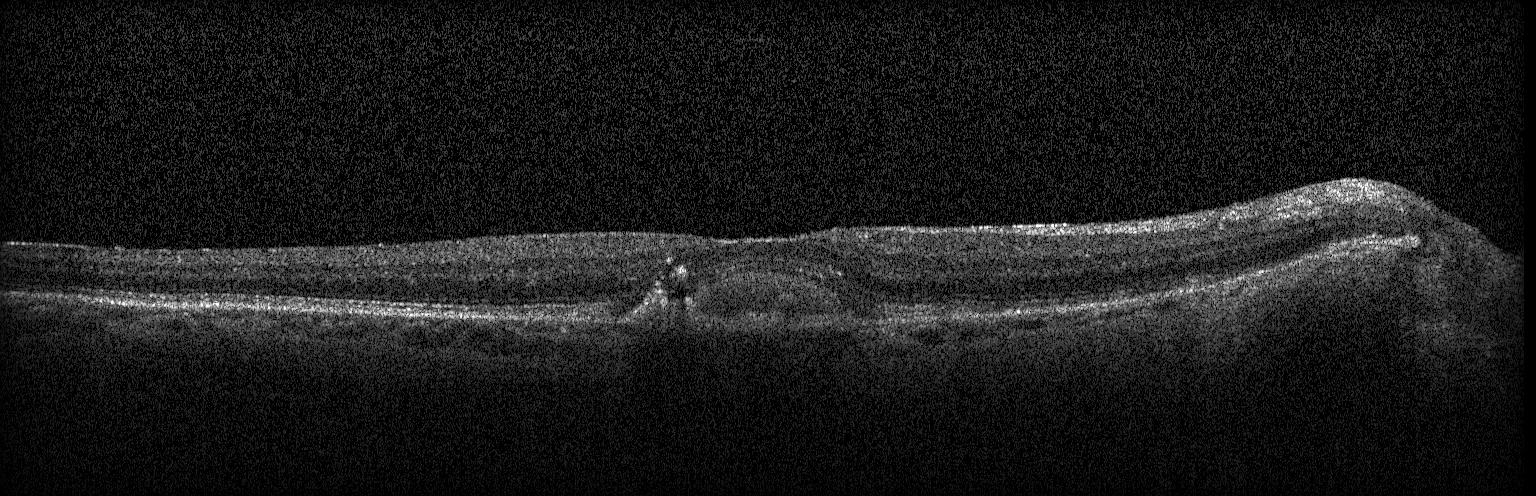

Acquired on a Heidelberg Spectralis. Fovea-centered. SD-OCT. OCT B-scan. Diagnosis: a choroidal neovascular membrane.